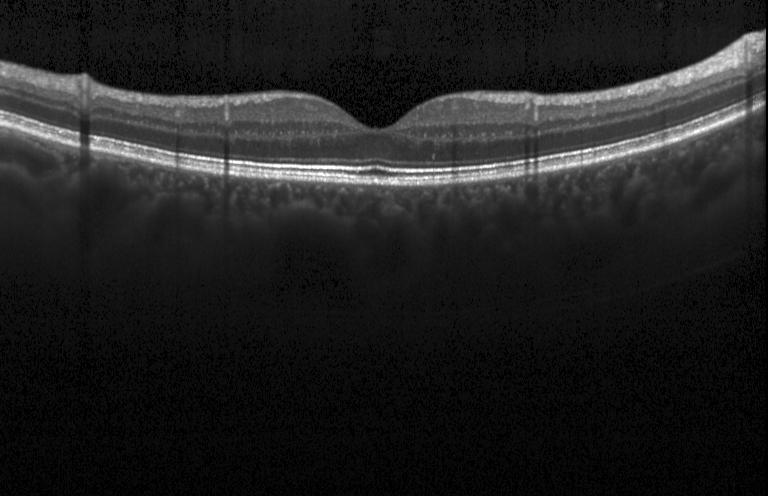 Retinal OCT cross-section, Heidelberg Spectralis OCT system, macular scan, SD-OCT. Impression: no evidence of choroidal neovascularization, diabetic macular edema, or drusen.